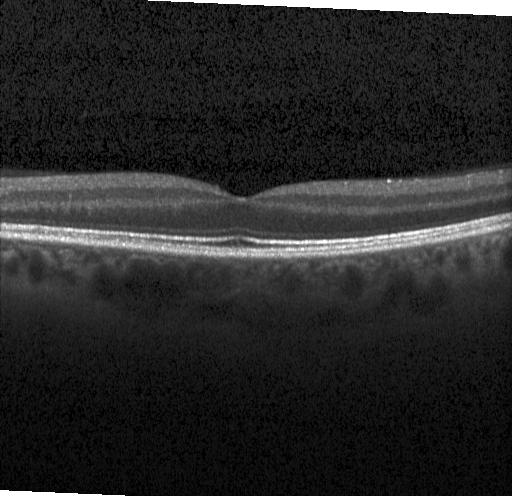

Retinal OCT B-scan, SD-OCT, Heidelberg Spectralis OCT system
Finding: no choroidal neovascularization, no diabetic macular edema, and no drusen.